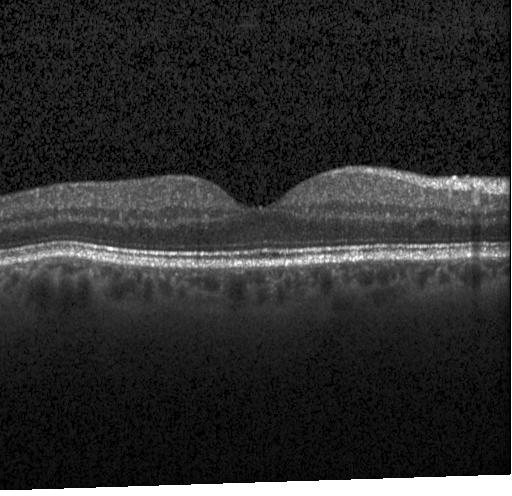 OCT B-scan. Horizontal scan through the fovea. Finding: no CNV, no DME, and no drusen.